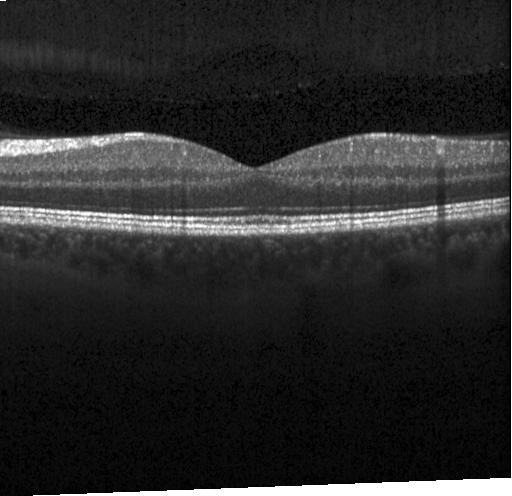

Heidelberg Spectralis OCT system; optical coherence tomography scan; horizontal scan through the fovea
Impression: neither choroidal neovascularization, diabetic macular edema, nor drusen.